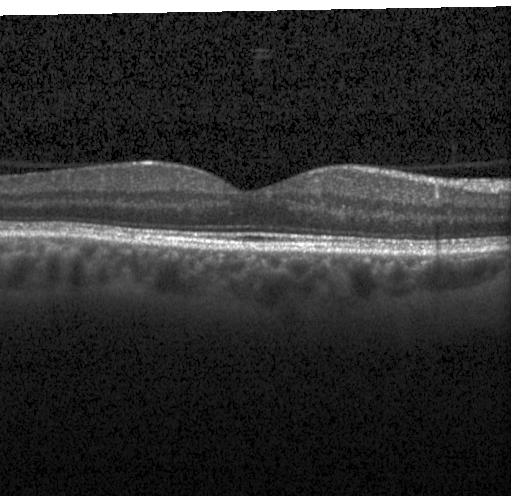 OCT B-scan.
Macular OCT: no evidence of choroidal neovascularization, diabetic macular edema, or drusen.